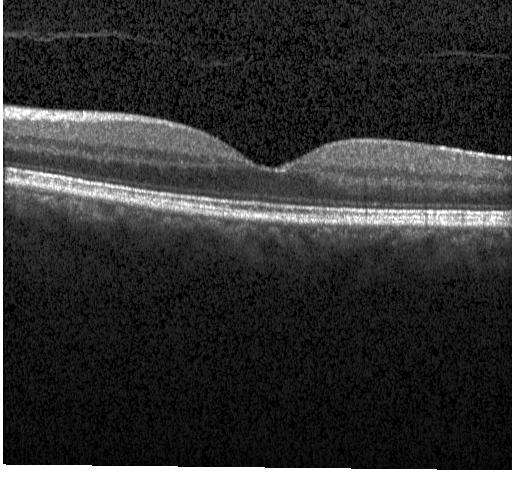

OCT B-scan · instrument: Heidelberg Spectralis · macular scan · SD-OCT.
OCT finding: neither choroidal neovascularization, diabetic macular edema, nor drusen.